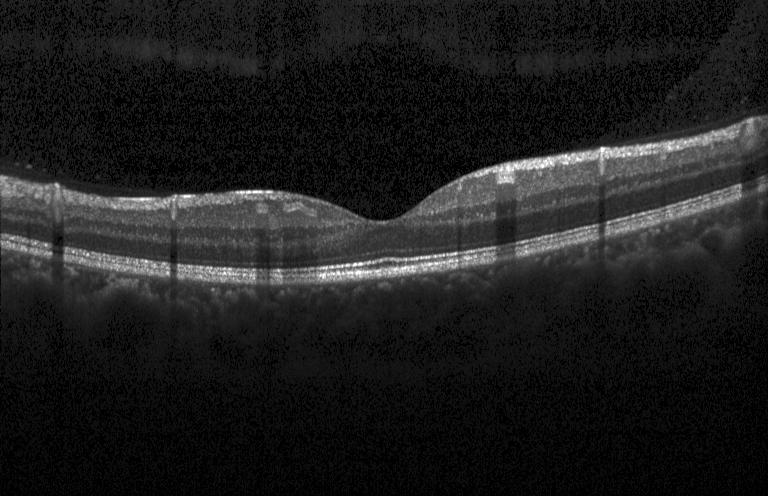
Retinal OCT cross-section. Acquired on a Heidelberg Spectralis. No choroidal neovascularization, no diabetic macular edema, and no drusen.